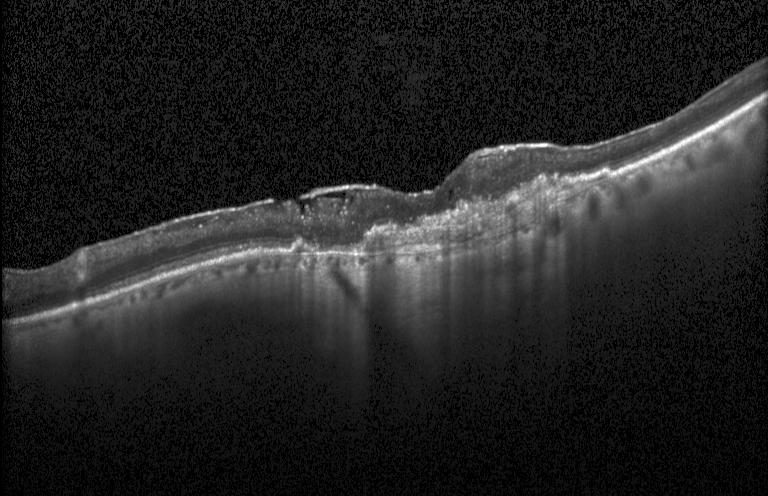
Spectral-domain optical coherence tomography; instrument: Heidelberg Spectralis; optical coherence tomography B-scan; through the macula — This B-scan demonstrates a choroidal neovascular membrane.